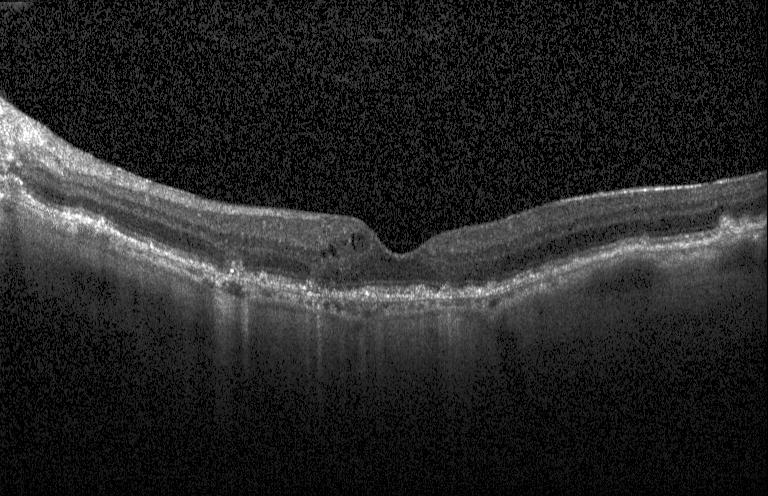 OCT scan showing a choroidal neovascular membrane.